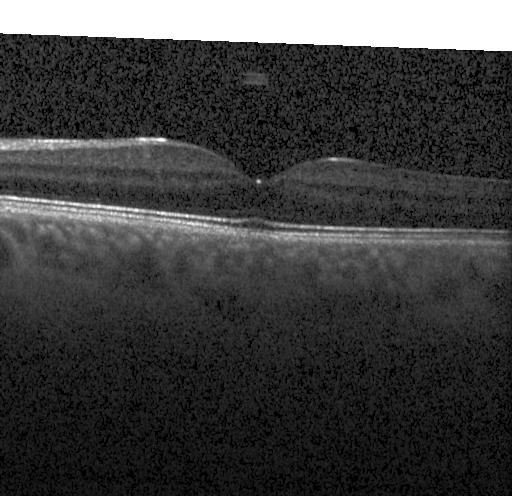

Spectral-domain OCT B-scan: no choroidal neovascularization, diabetic macular edema, or drusen.